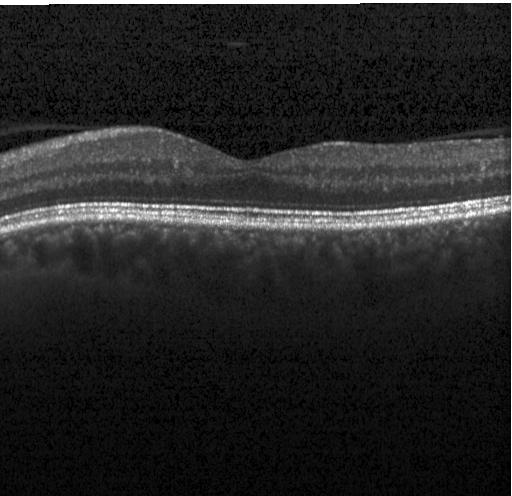 Spectral-domain OCT B-scan: no choroidal neovascularization, no diabetic macular edema, and no drusen.